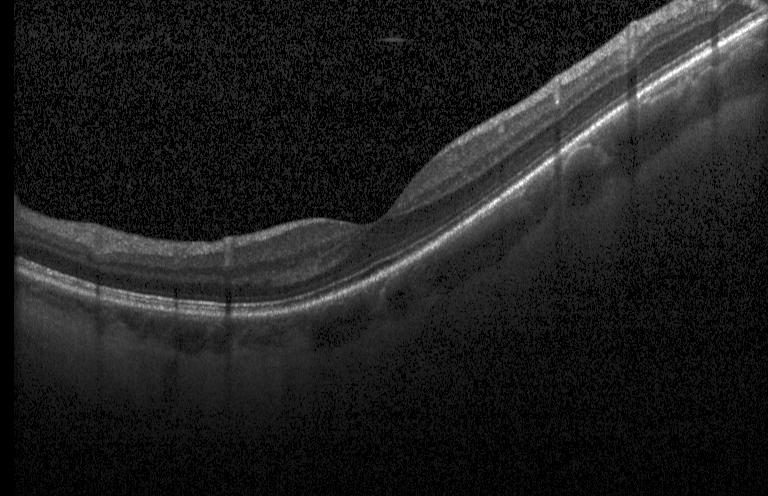
Finding: neither choroidal neovascularization, diabetic macular edema, nor drusen.